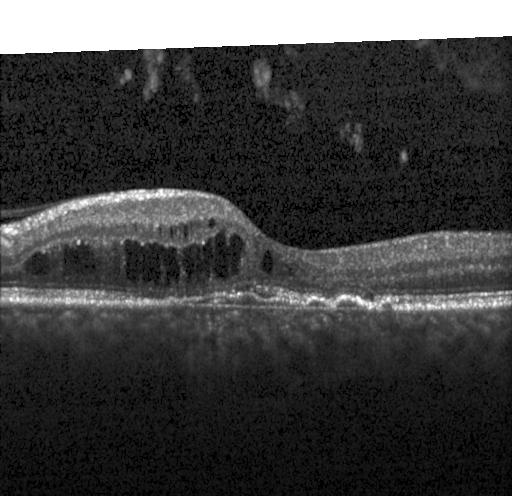 OCT finding: a choroidal neovascular membrane.